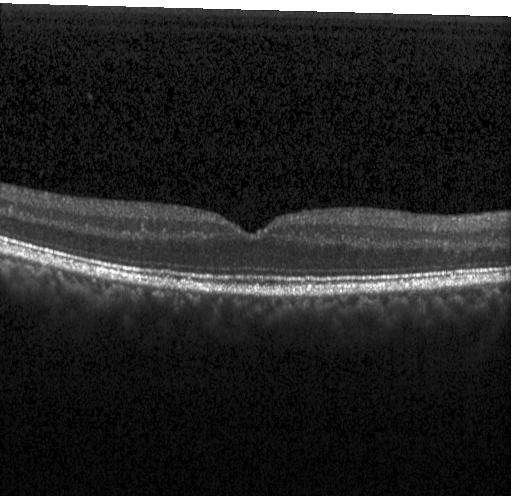

Finding: neither choroidal neovascularization, diabetic macular edema, nor drusen.